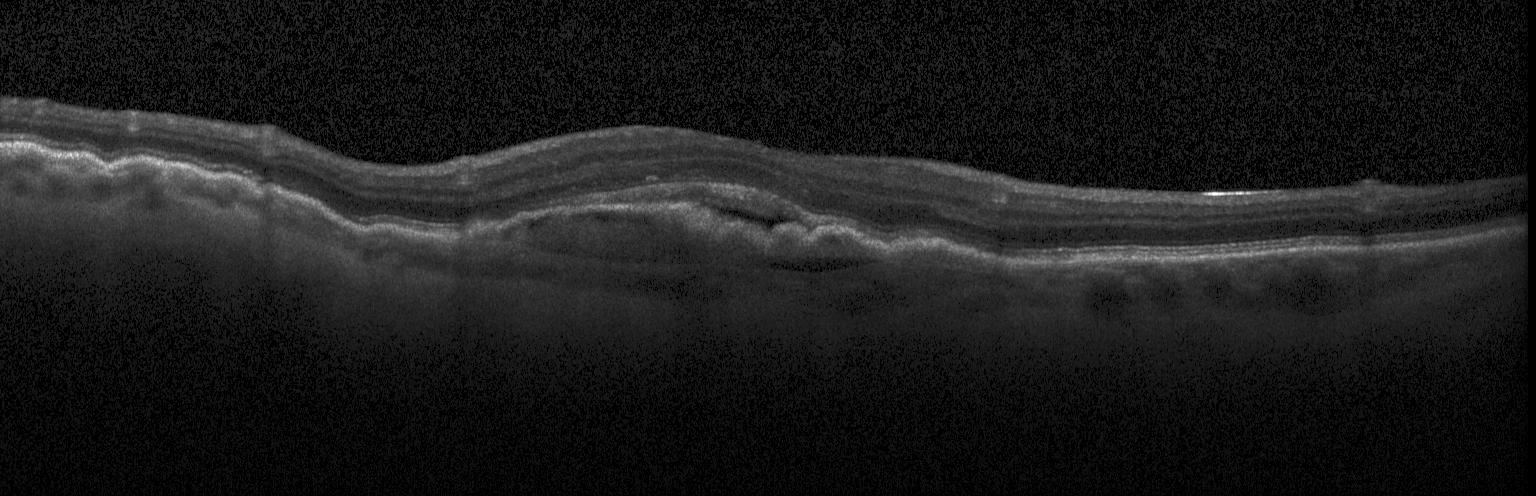
OCT finding: a choroidal neovascular membrane.